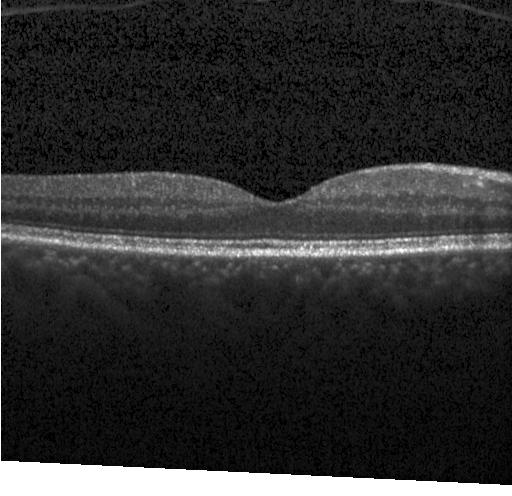 Instrument: Heidelberg Spectralis. OCT B-scan — Neither CNV, DME, nor drusen.